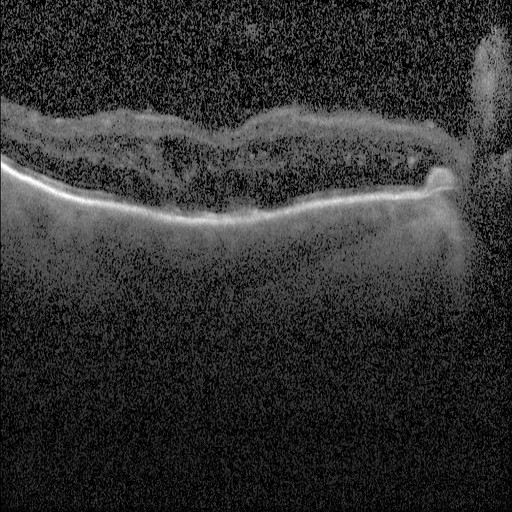
Heidelberg Spectralis. Optical coherence tomography B-scan.
Dx: diabetic macular edema.